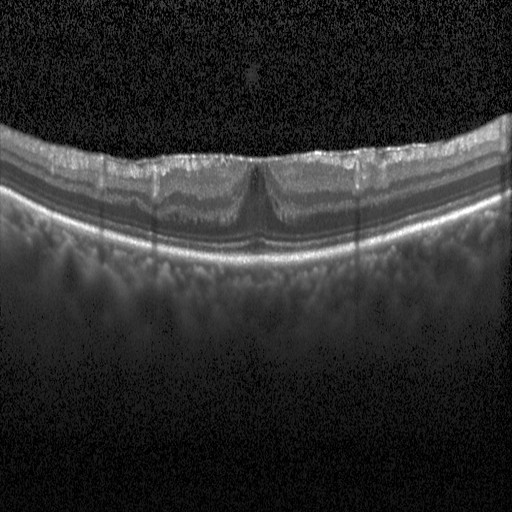 Finding: diabetic macular edema.